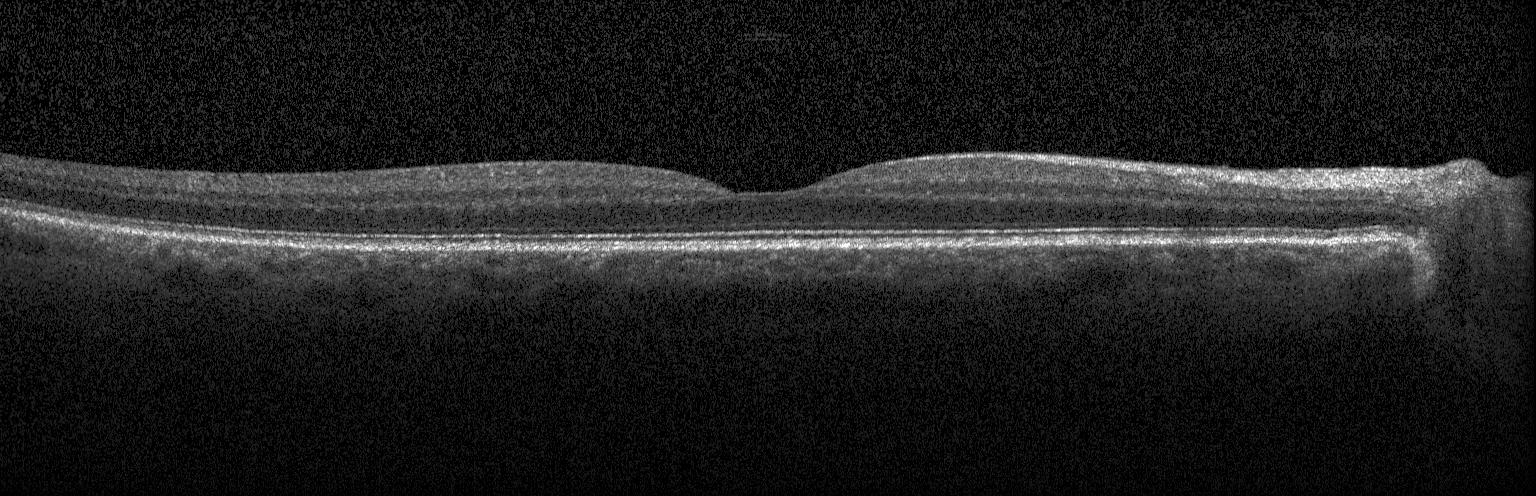
Optical coherence tomography scan · centered on the fovea · Heidelberg Spectralis OCT system · spectral-domain OCT. Impression: neither choroidal neovascularization, diabetic macular edema, nor drusen.